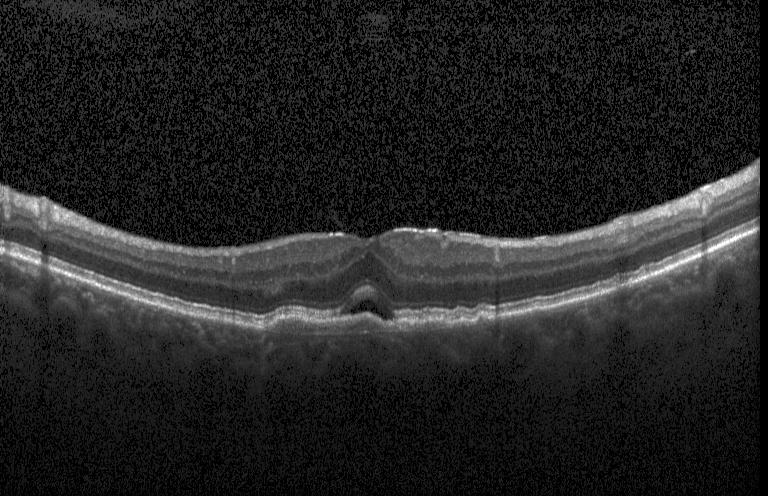 Retinal OCT cross-section — Diagnosis: a choroidal neovascular membrane.